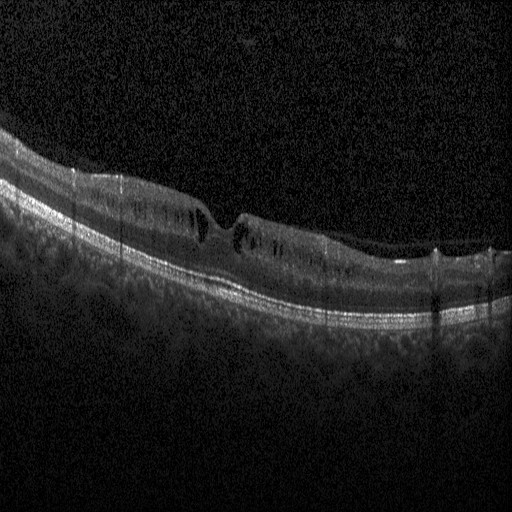

Through the macula; optical coherence tomography scan; instrument: Heidelberg Spectralis. OCT finding: DME.